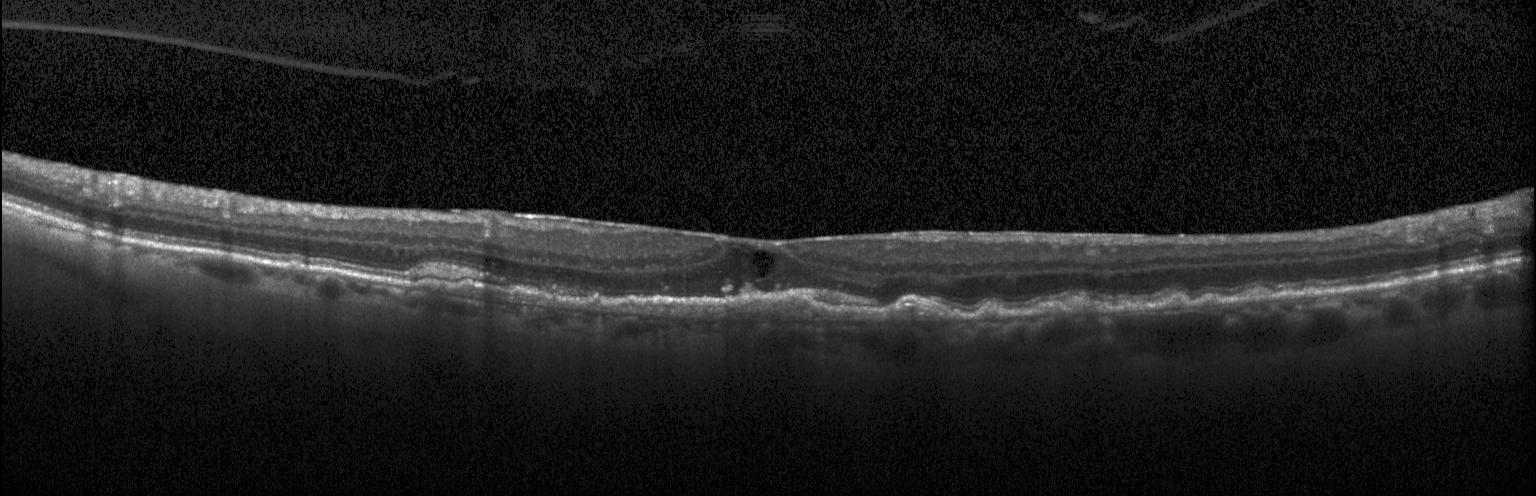 Impression: a choroidal neovascular membrane.